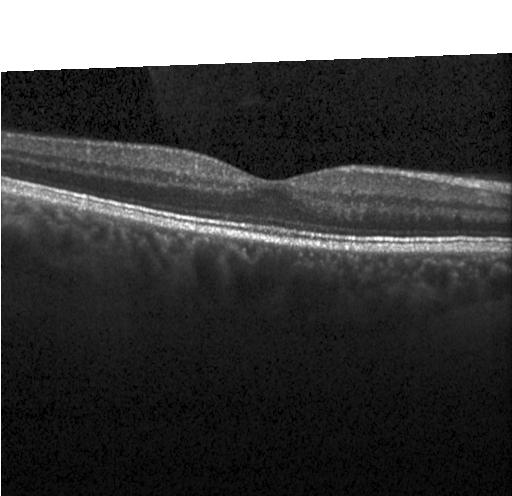
Heidelberg Spectralis OCT system. Optical coherence tomography B-scan. Through the macula.
Diagnosis: neither choroidal neovascularization, diabetic macular edema, nor drusen.